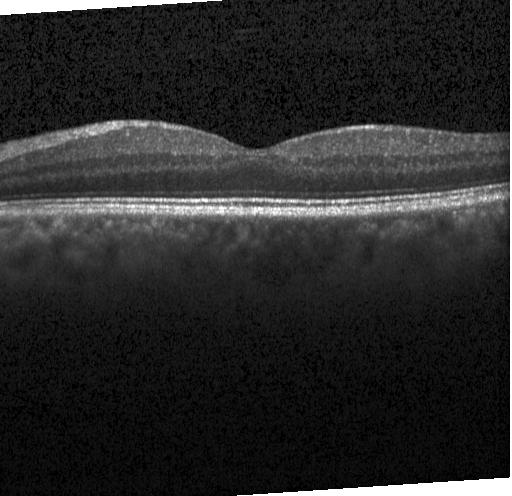
Acquired on a Heidelberg Spectralis · macular scan · optical coherence tomography scan.
Dx: no choroidal neovascularization, no diabetic macular edema, and no drusen.